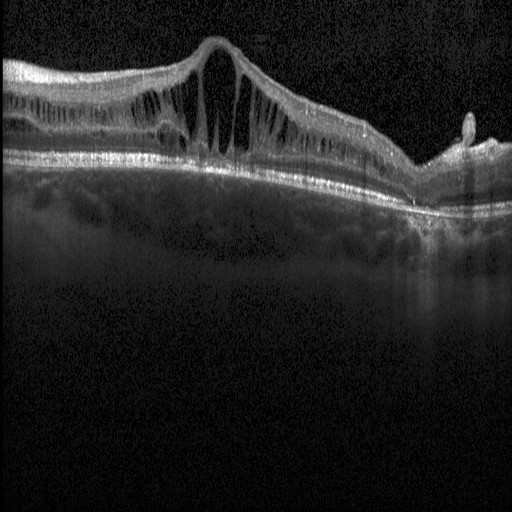

Centered on the fovea · retinal OCT B-scan · spectral-domain optical coherence tomography. Impression: DME.